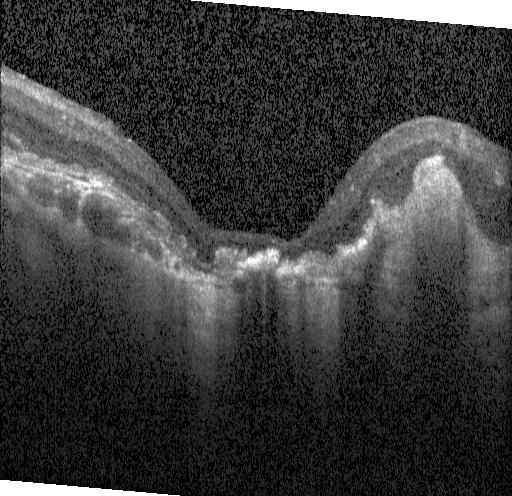
Optical coherence tomography B-scan; horizontal scan through the fovea; spectral-domain OCT.
Choroidal neovascularization.